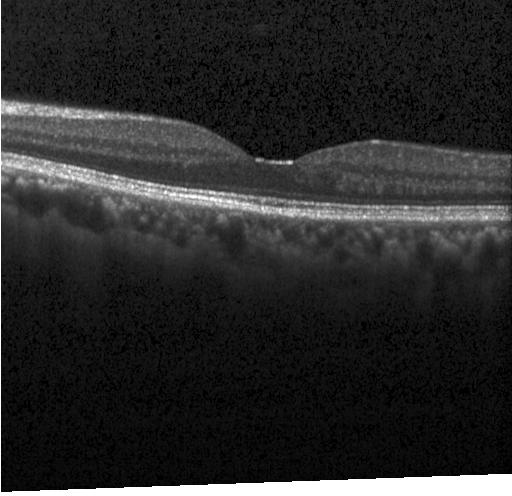 Diagnosis: neither choroidal neovascularization, diabetic macular edema, nor drusen.